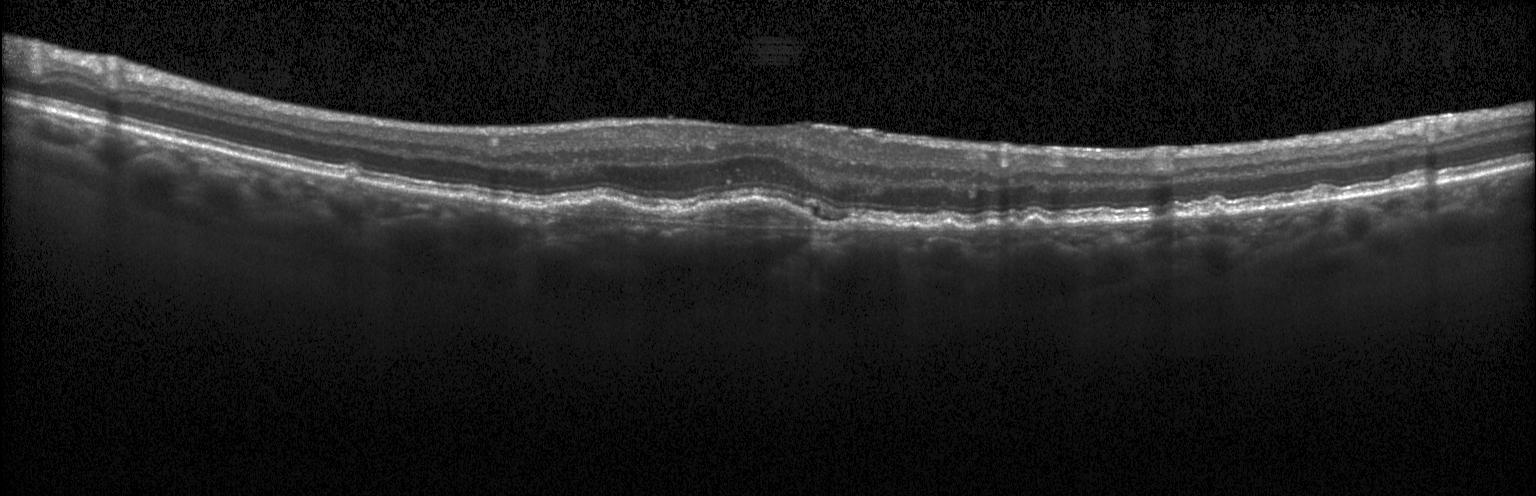
OCT line scan; Heidelberg Spectralis; horizontal scan through the fovea.
Diagnosis: choroidal neovascularization.